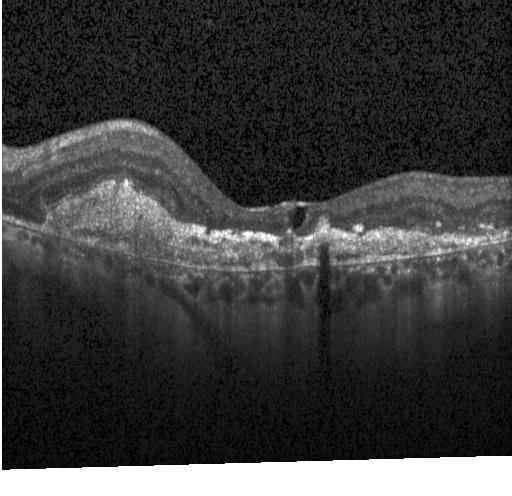
Retinal OCT cross-section, SD-OCT
Assessment: choroidal neovascularization.